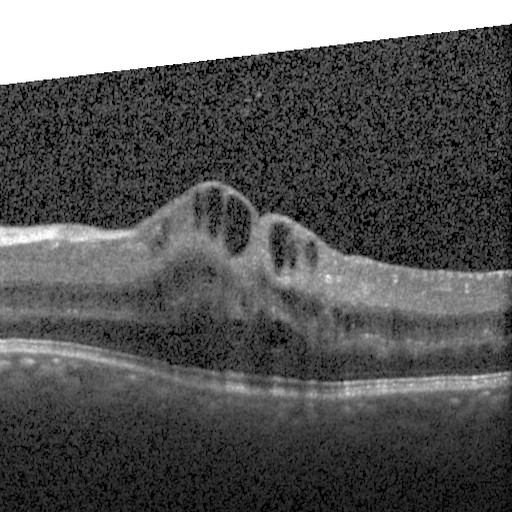

OCT B-scan.
Impression: diabetic macular edema.